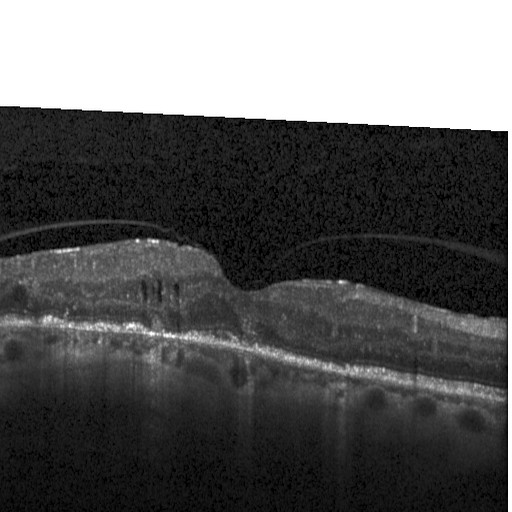

Macular OCT demonstrating diabetic macular edema.